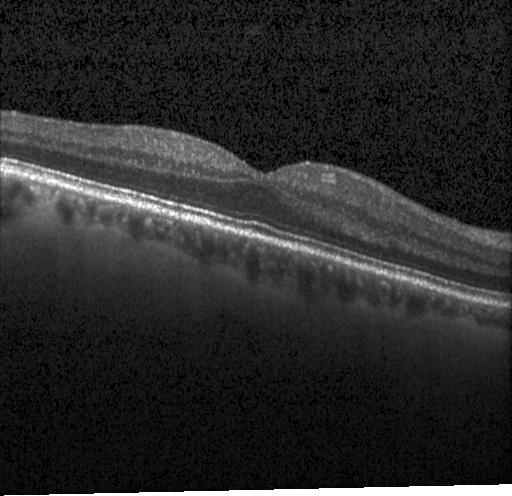 Finding: no choroidal neovascularization, diabetic macular edema, or drusen.